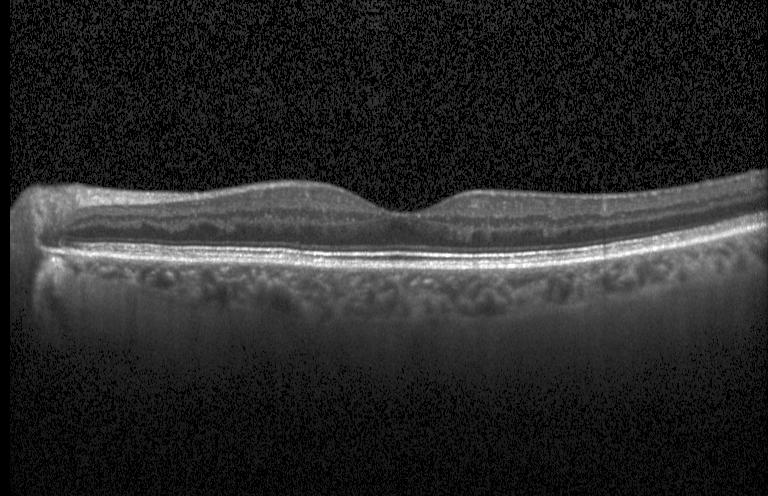

Retinal OCT B-scan — This B-scan demonstrates no choroidal neovascularization, diabetic macular edema, or drusen.